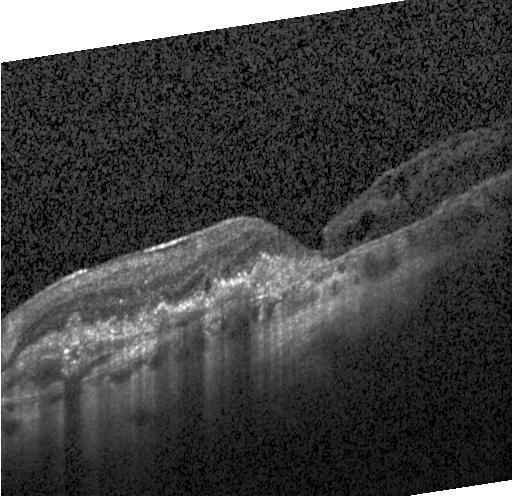
Retinal OCT B-scan, instrument: Heidelberg Spectralis.
Finding: CNV.